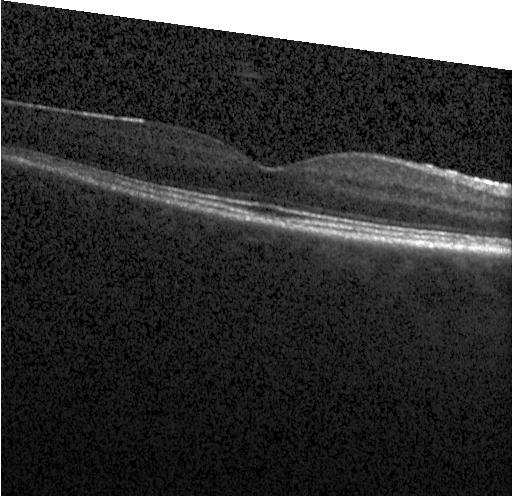

Macular scan. Optical coherence tomography B-scan.
Finding: no choroidal neovascularization, diabetic macular edema, or drusen.